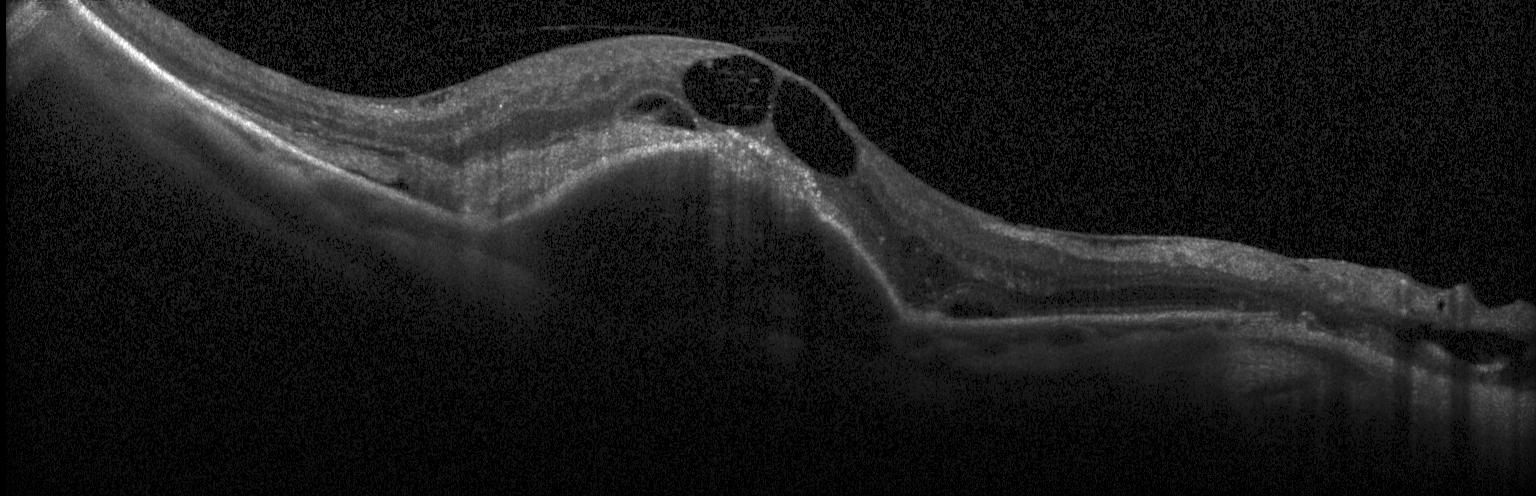
Diagnosis: a choroidal neovascular membrane.